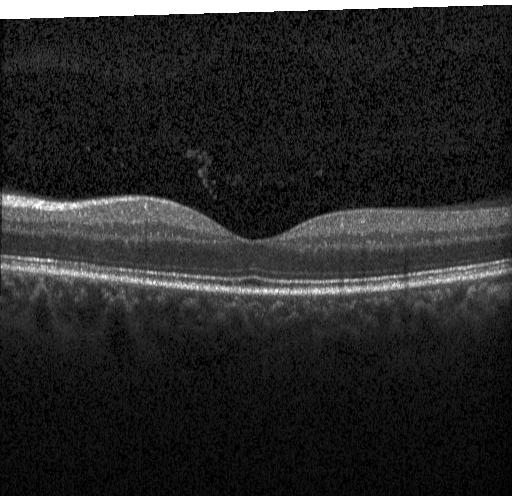

Instrument: Heidelberg Spectralis; fovea-centered; OCT B-scan; spectral-domain optical coherence tomography. Finding: neither choroidal neovascularization, diabetic macular edema, nor drusen.